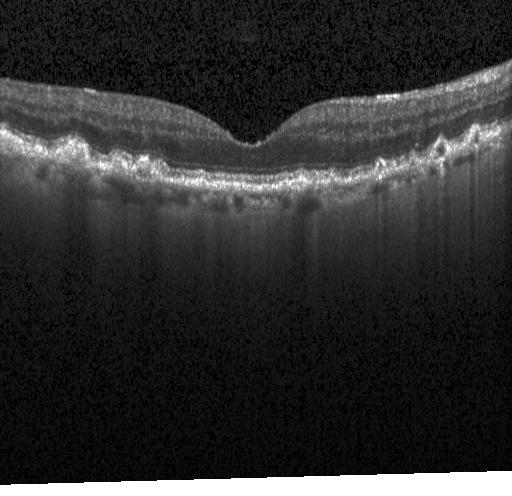 Multiple drusen.